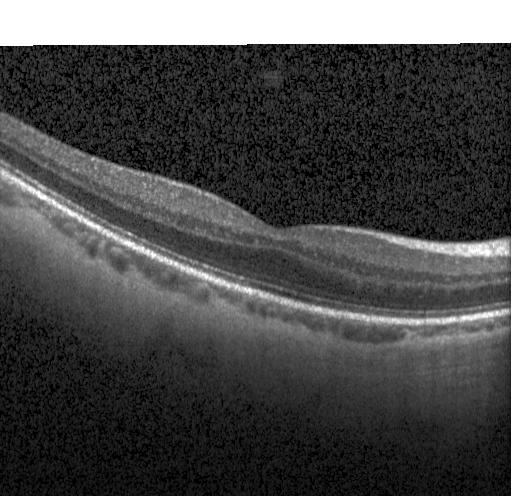 Through the macula, optical coherence tomography B-scan — The scan shows no choroidal neovascularization, diabetic macular edema, or drusen.